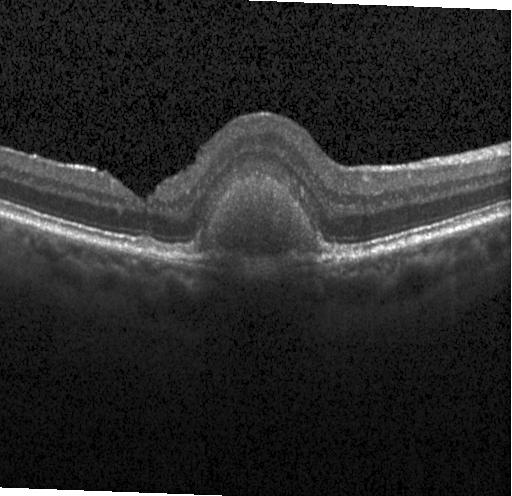
SD-OCT; OCT B-scan; instrument: Heidelberg Spectralis; centered on the fovea.
Diagnosis: CNV.